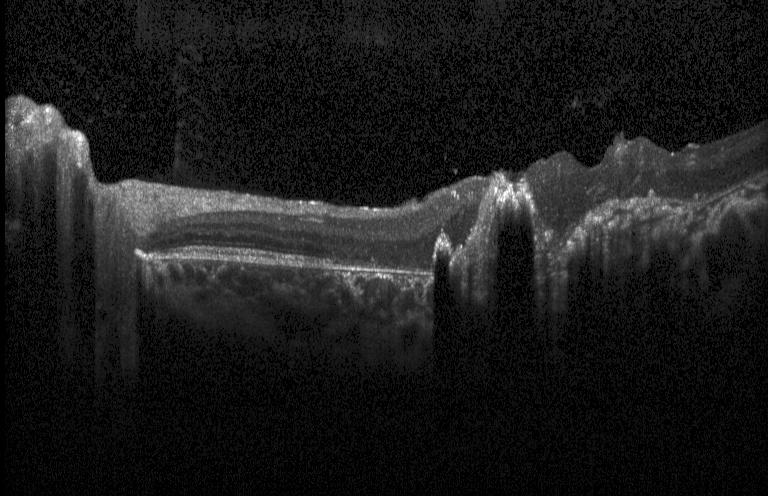

OCT scan showing a choroidal neovascular membrane.